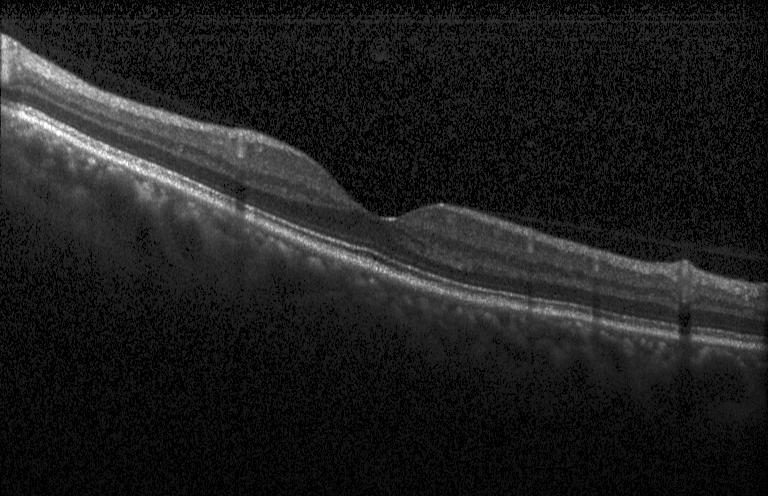 Dx: neither choroidal neovascularization, diabetic macular edema, nor drusen.